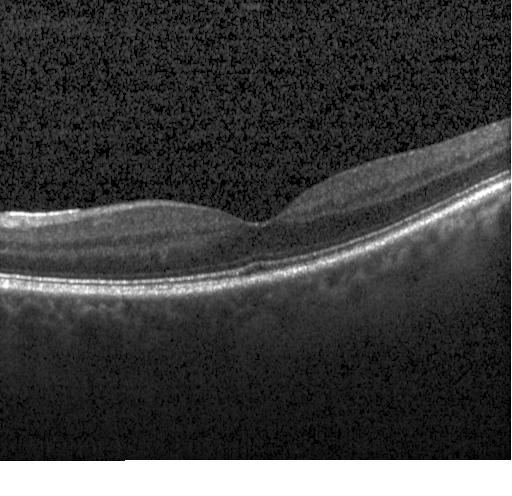 OCT finding: neither choroidal neovascularization, diabetic macular edema, nor drusen.